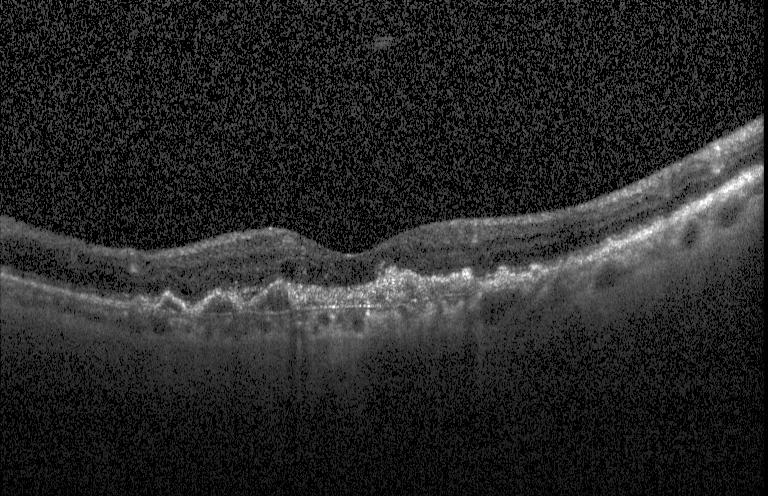 Dx: choroidal neovascularization (CNV).